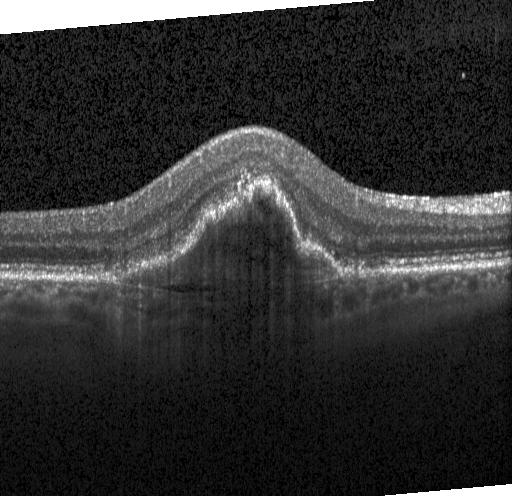

Retinal OCT cross-section. Acquired on a Heidelberg Spectralis. SD-OCT. Macular scan
Choroidal neovascularization (CNV).